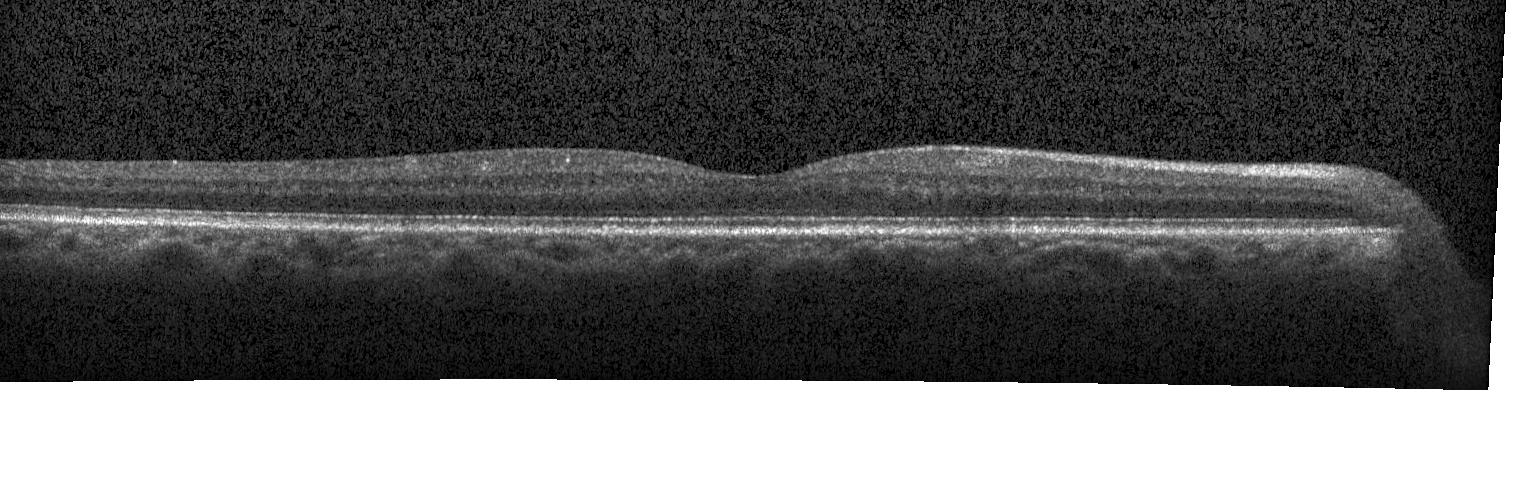
OCT B-scan.
Impression: no choroidal neovascularization, diabetic macular edema, or drusen.